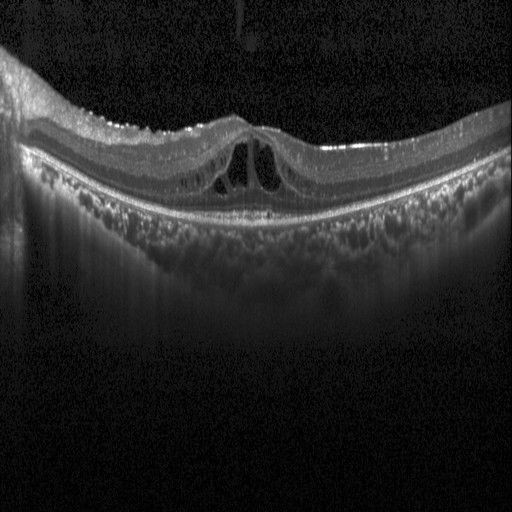
Spectral-domain OCT B-scan: DME.